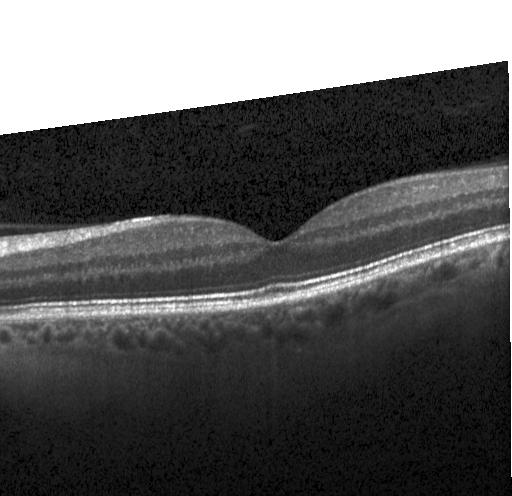 Horizontal scan through the fovea. Spectral-domain OCT. Retinal OCT B-scan. Acquired on a Heidelberg Spectralis. The scan shows no evidence of CNV, DME, or drusen.